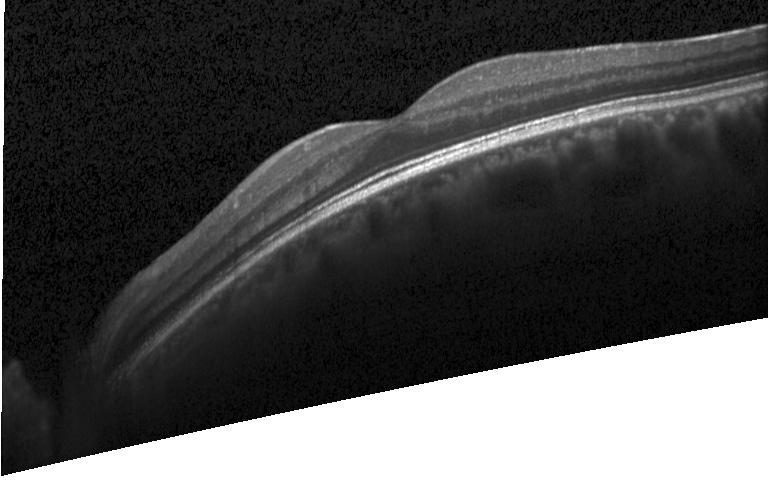
Centered on the fovea · Heidelberg Spectralis · optical coherence tomography B-scan · spectral-domain OCT.
OCT finding: no evidence of choroidal neovascularization, diabetic macular edema, or drusen.